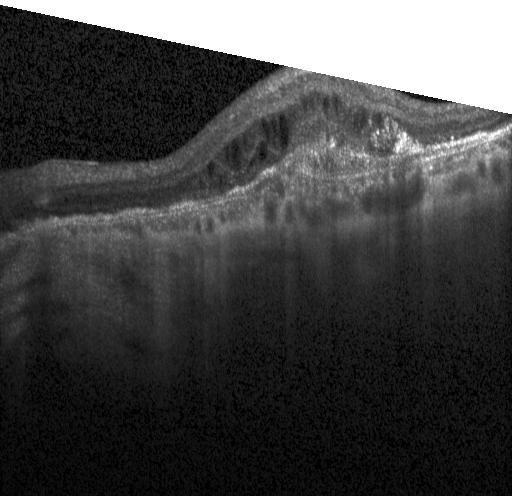
Retinal OCT B-scan
Finding: a choroidal neovascular membrane.